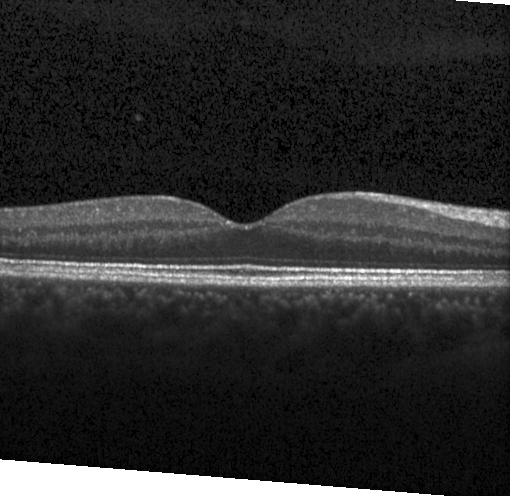 Dx: no evidence of CNV, DME, or drusen.